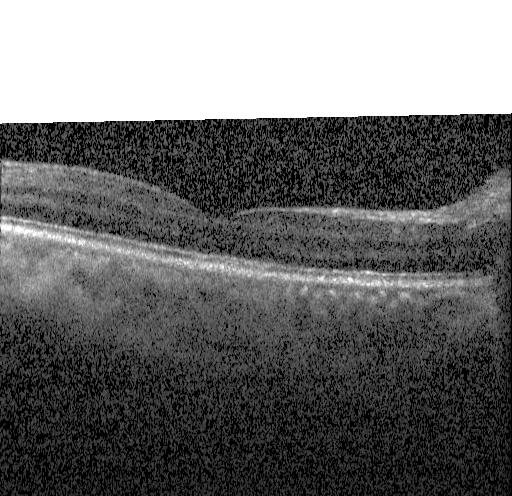
Acquired on a Heidelberg Spectralis; macular scan; retinal OCT B-scan.
Assessment: neither choroidal neovascularization, diabetic macular edema, nor drusen.